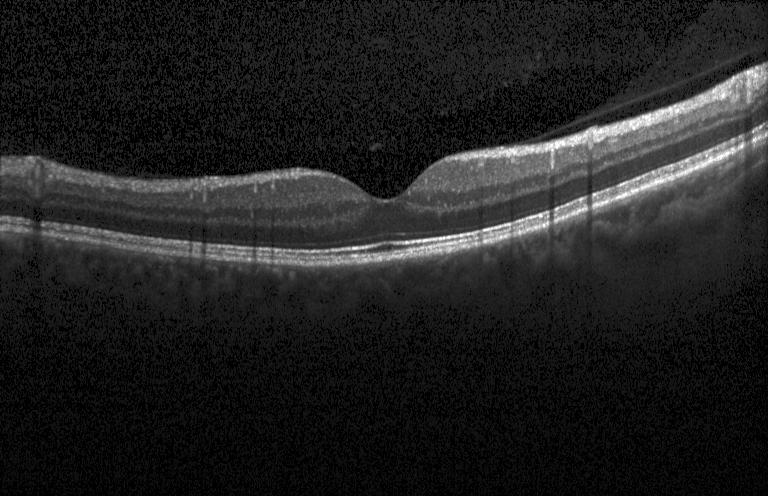

Retinal OCT cross-section; acquired on a Heidelberg Spectralis; spectral-domain OCT; through the macula. Impression: no choroidal neovascularization, no diabetic macular edema, and no drusen.